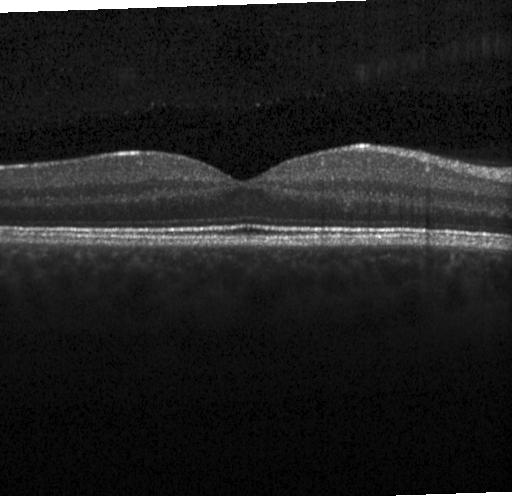 Instrument: Heidelberg Spectralis; retinal OCT cross-section
No choroidal neovascularization, no diabetic macular edema, and no drusen.